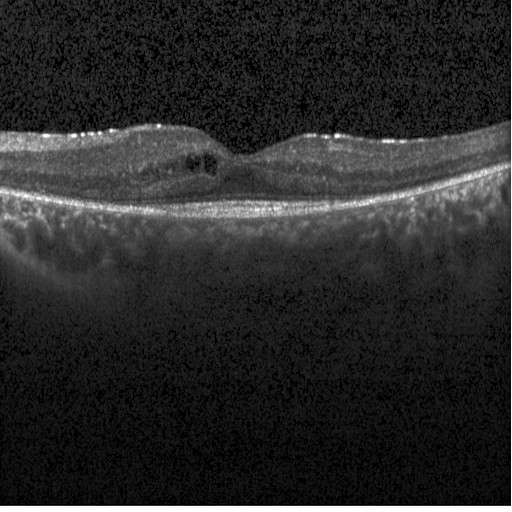 Assessment: DME.